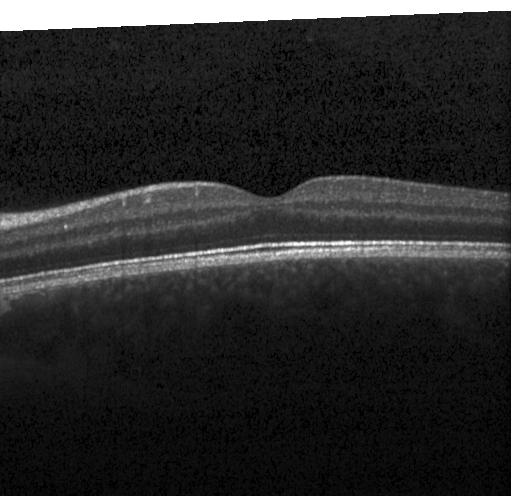

Heidelberg Spectralis OCT system; OCT line scan; horizontal scan through the fovea.
No choroidal neovascularization, no diabetic macular edema, and no drusen.